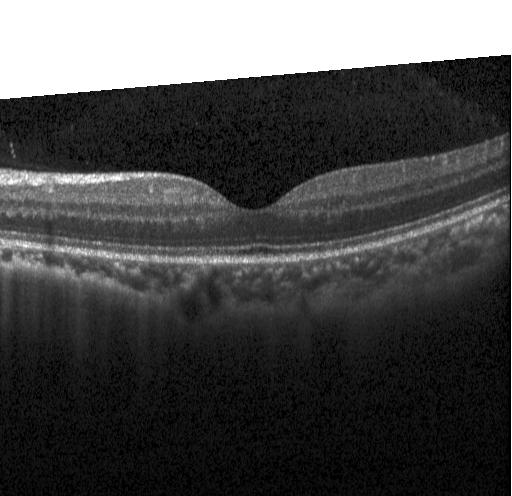

Finding: neither choroidal neovascularization, diabetic macular edema, nor drusen.